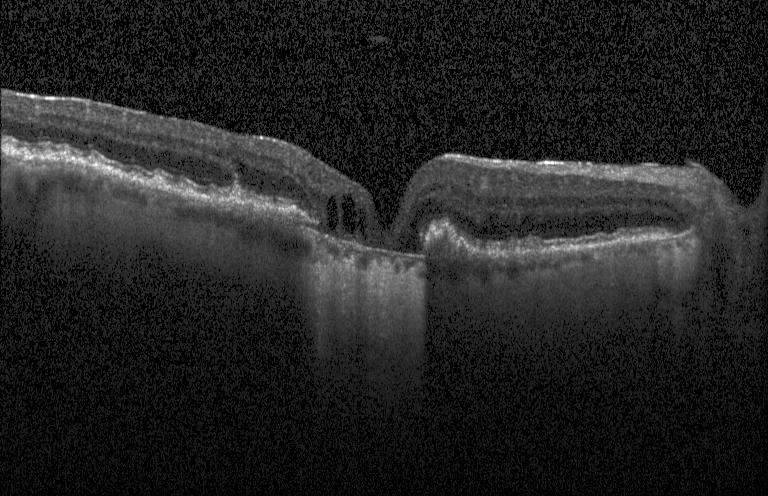
Macular OCT demonstrating a choroidal neovascular membrane.